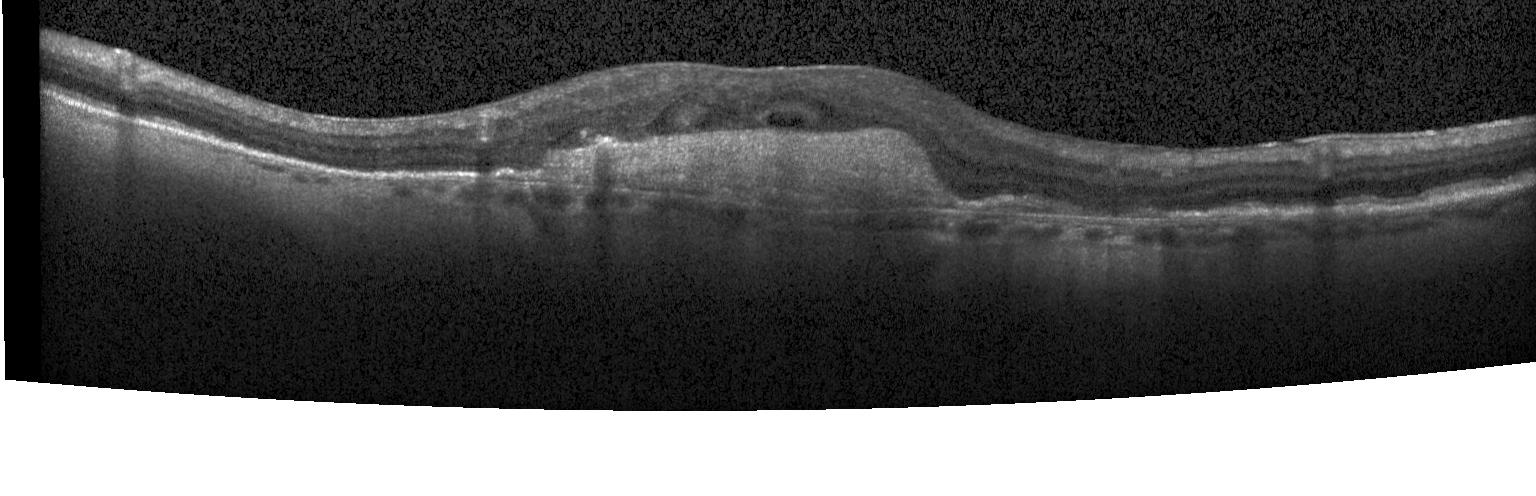

OCT line scan; spectral-domain optical coherence tomography; Heidelberg Spectralis; macular scan — Finding: CNV.